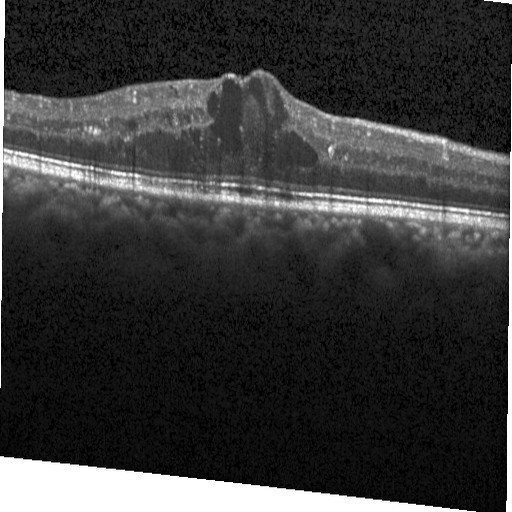

OCT line scan. Centered on the fovea. Instrument: Heidelberg Spectralis
Finding: DME.